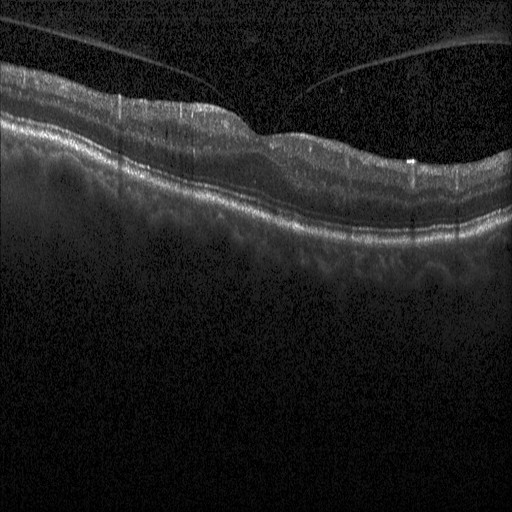

OCT scan showing diabetic macular edema (DME).